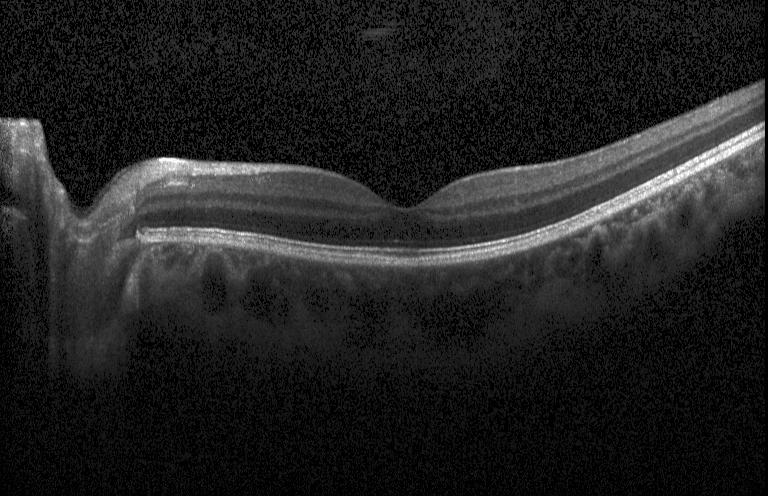

Macular OCT demonstrating no evidence of CNV, DME, or drusen.